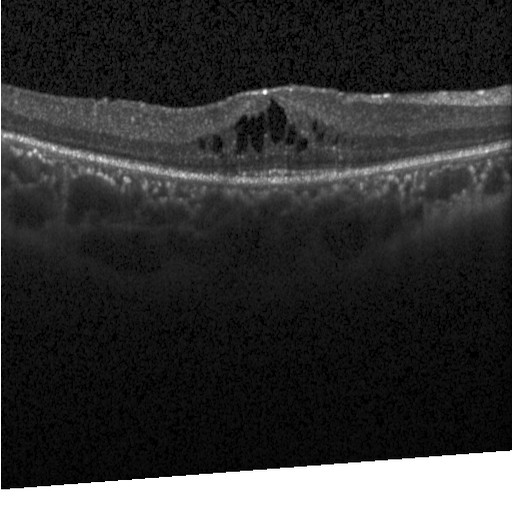
Assessment: DME.